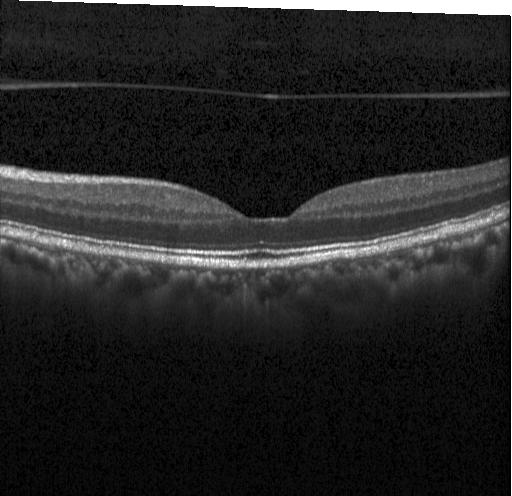 Heidelberg Spectralis; optical coherence tomography B-scan.
Impression: no choroidal neovascularization, diabetic macular edema, or drusen.